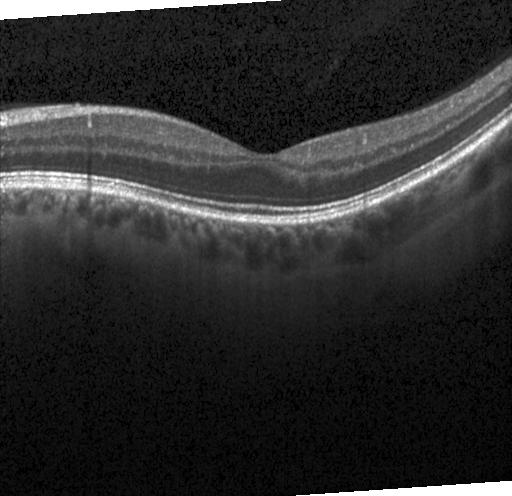

Finding: neither choroidal neovascularization, diabetic macular edema, nor drusen.